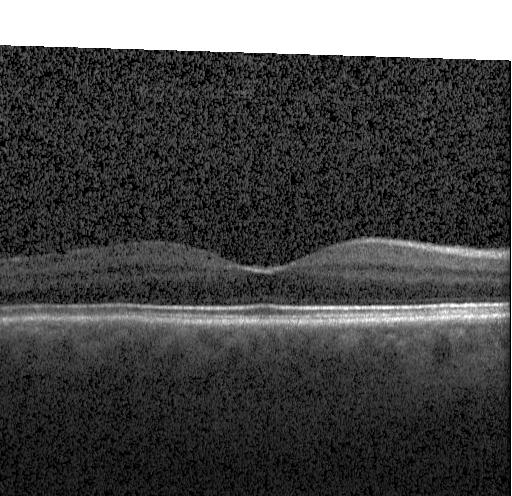

Optical coherence tomography scan
No evidence of choroidal neovascularization, diabetic macular edema, or drusen.